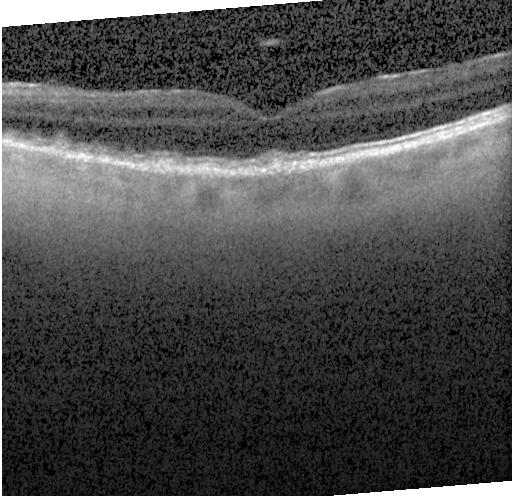 The scan shows multiple drusen.